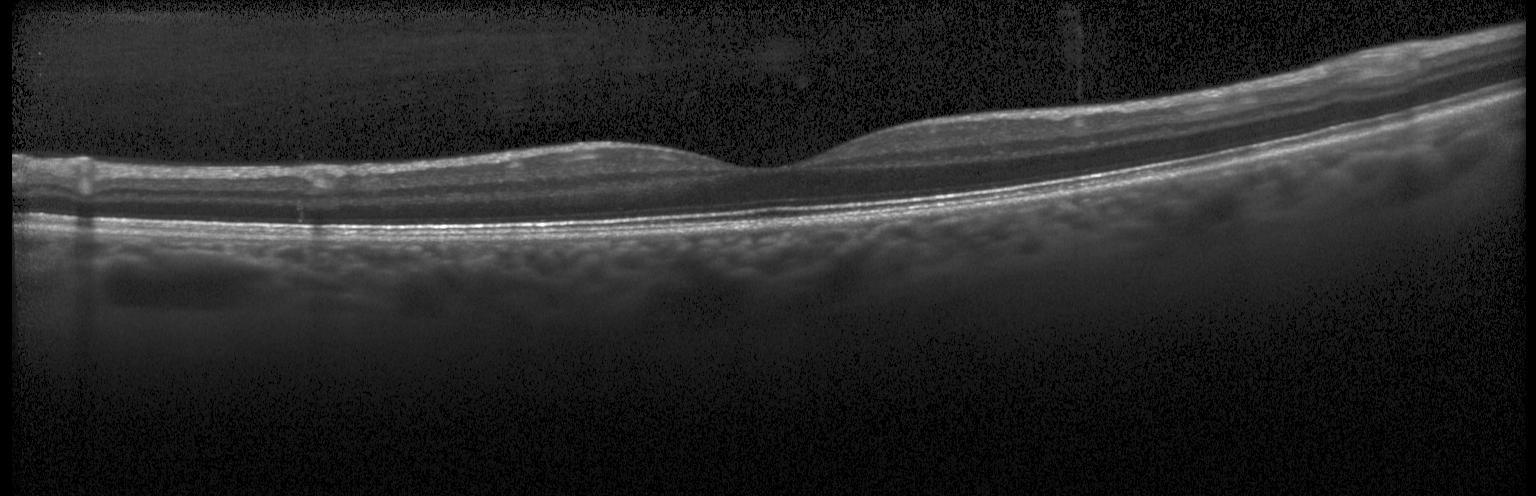
Optical coherence tomography scan. Heidelberg Spectralis. SD-OCT. Dx: no choroidal neovascularization, no diabetic macular edema, and no drusen.